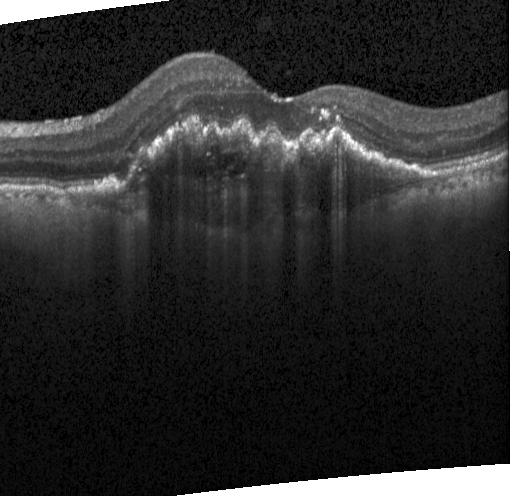

Retinal OCT cross-section showing a choroidal neovascular membrane.